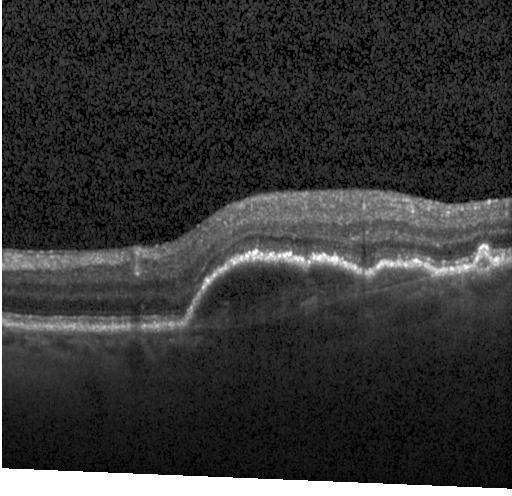
Finding: a choroidal neovascular membrane.